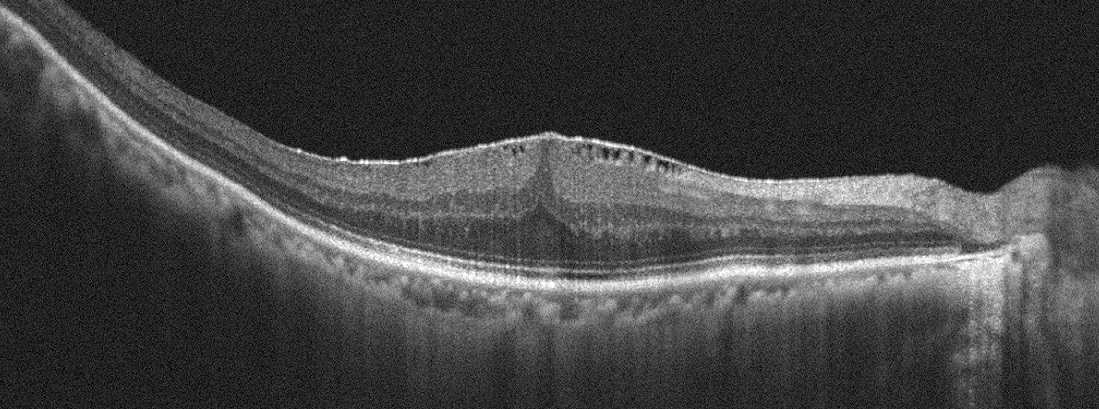

OCT B-scan; macular scan; instrument: Optovue Avanti RTVue XR.
The scan shows ERM.